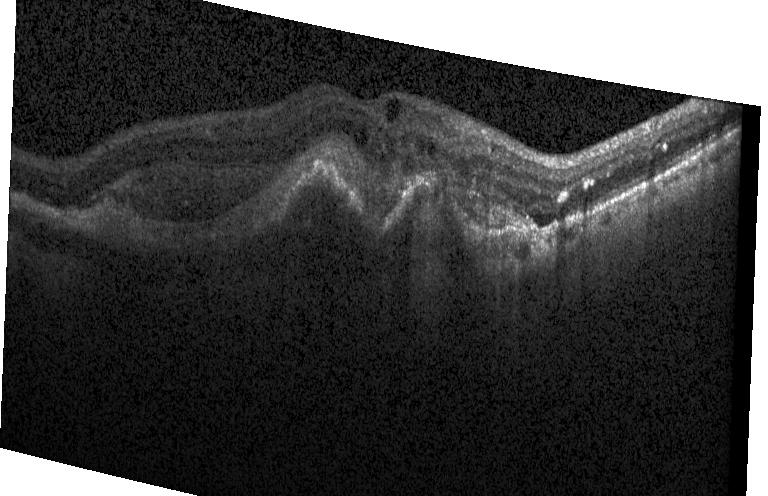

Impression: a choroidal neovascular membrane.